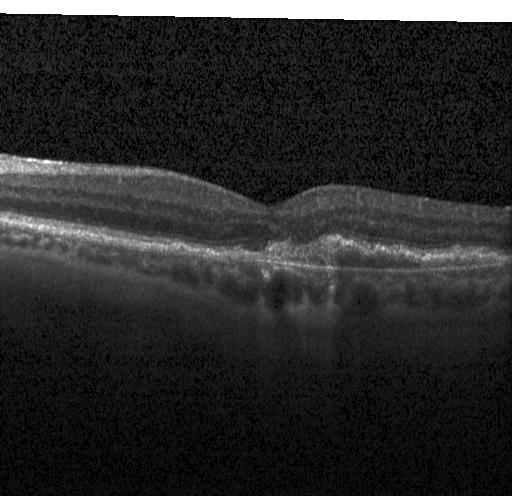
Retinal OCT B-scan. Heidelberg Spectralis. SD-OCT — Choroidal neovascularization.